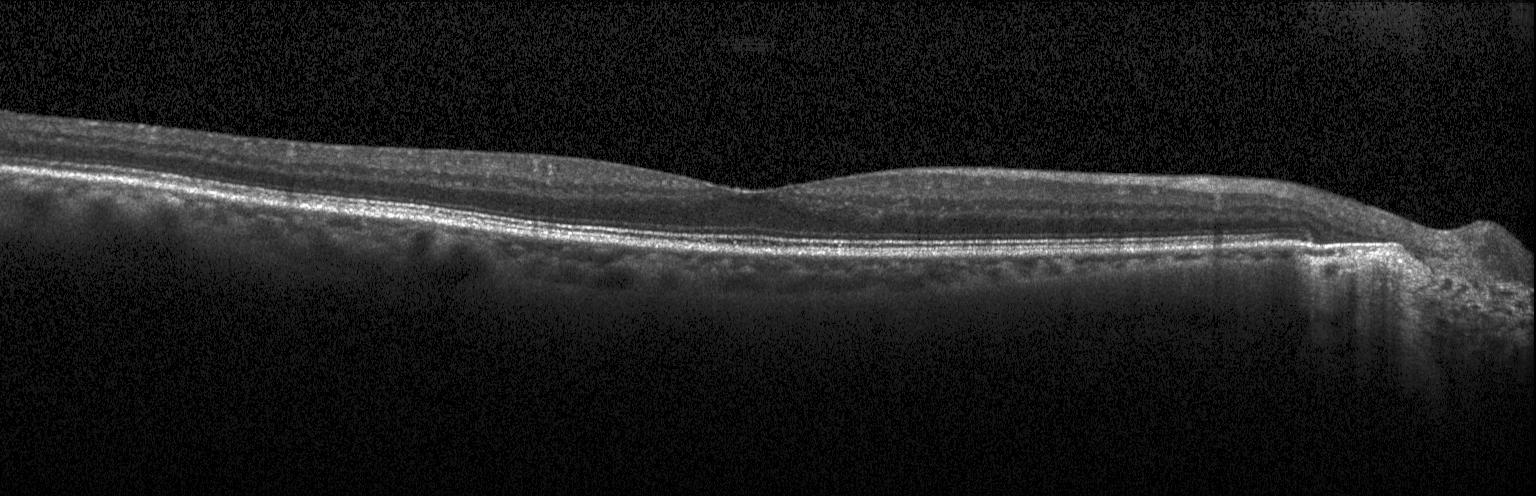
Spectral-domain OCT. Heidelberg Spectralis OCT system. Fovea-centered. OCT B-scan
Impression: neither choroidal neovascularization, diabetic macular edema, nor drusen.